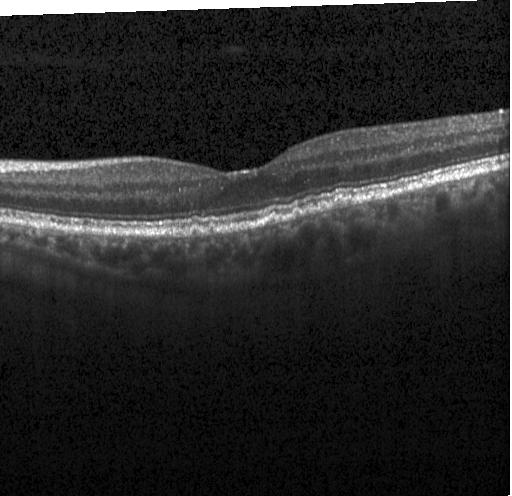
Optical coherence tomography scan · through the macula
This B-scan demonstrates sub-RPE drusenoid deposits.